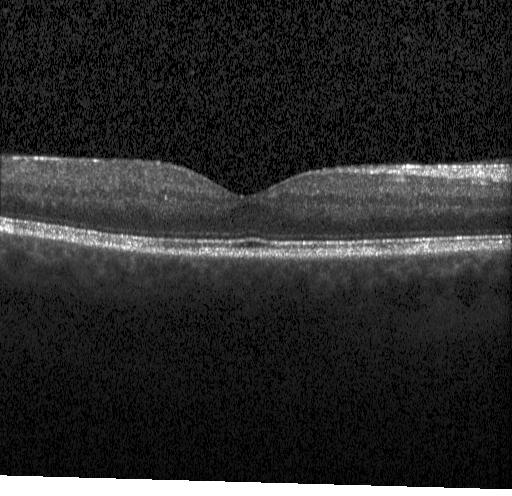

OCT finding: no choroidal neovascularization, diabetic macular edema, or drusen.